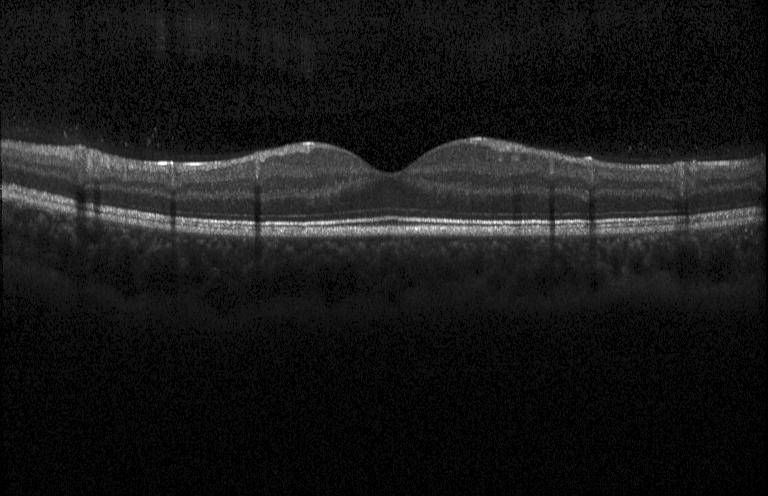 Finding: no choroidal neovascularization, diabetic macular edema, or drusen.